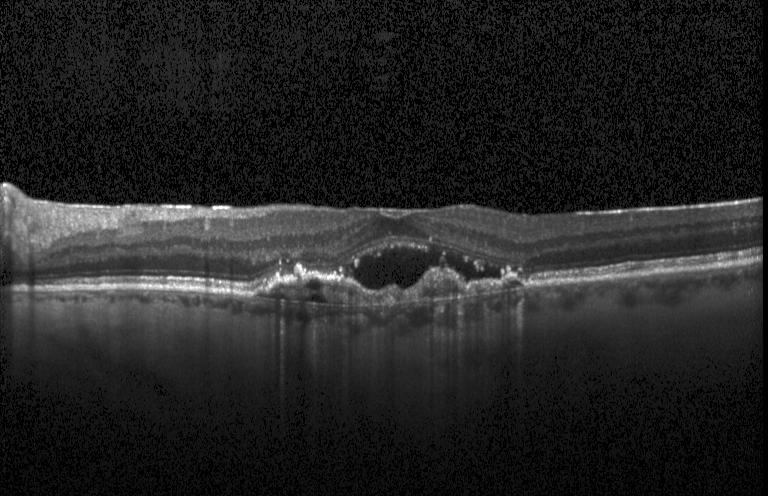

Centered on the fovea · instrument: Heidelberg Spectralis · retinal OCT cross-section
OCT finding: CNV.